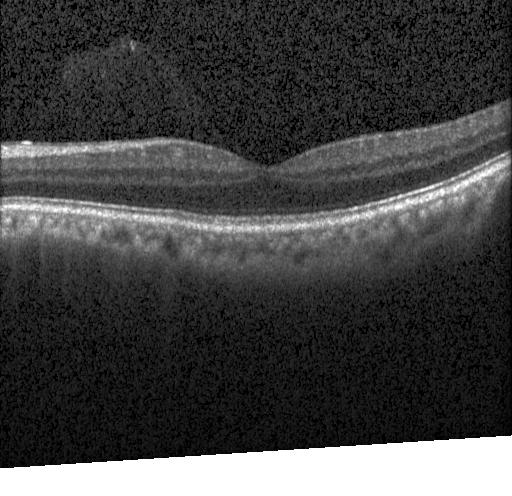
Retinal OCT cross-section showing no choroidal neovascularization, no diabetic macular edema, and no drusen.